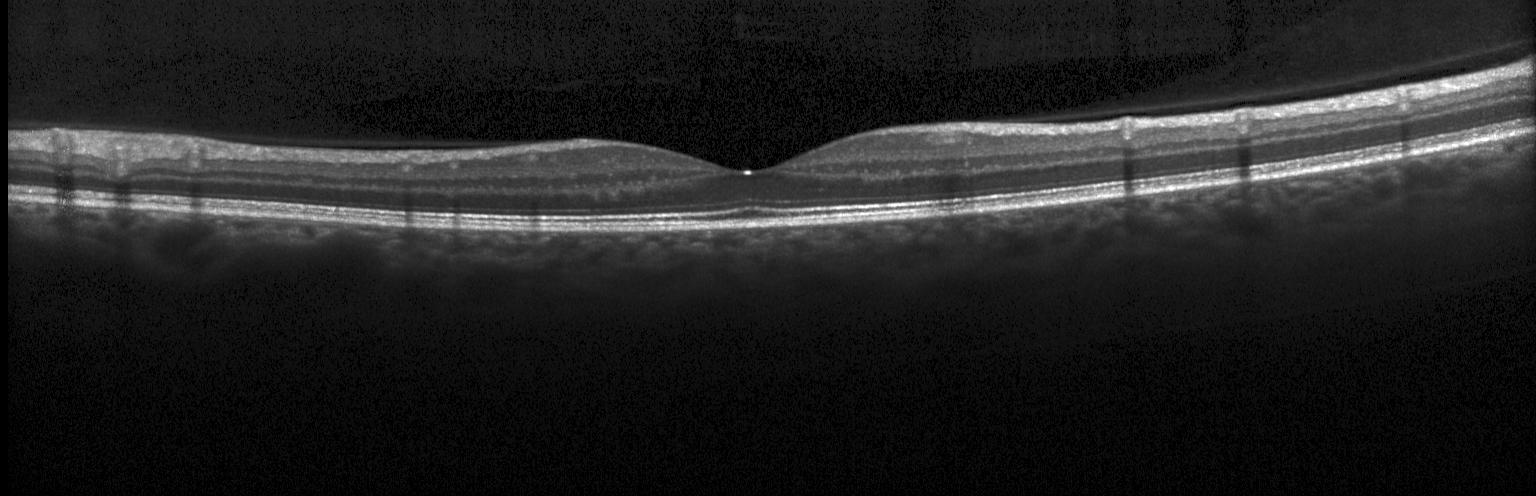

Horizontal scan through the fovea. Heidelberg Spectralis. OCT line scan. Spectral-domain OCT — Diagnosis: no choroidal neovascularization, diabetic macular edema, or drusen.